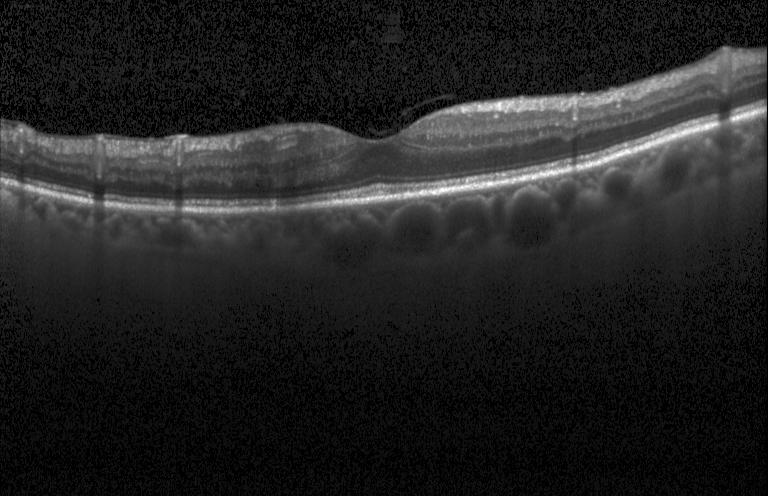
Finding: neither CNV, DME, nor drusen.